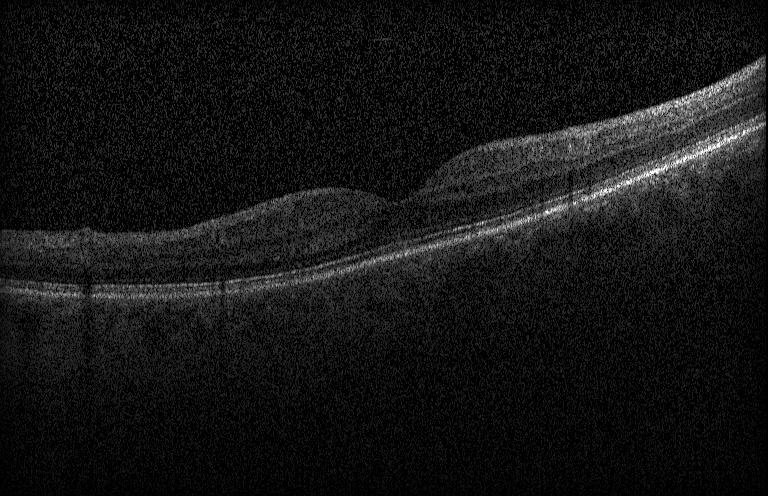
Impression: no evidence of choroidal neovascularization, diabetic macular edema, or drusen.